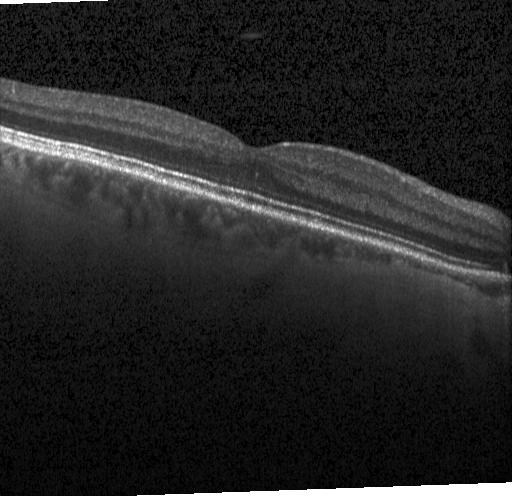
OCT B-scan; centered on the fovea; spectral-domain optical coherence tomography; instrument: Heidelberg Spectralis.
The scan shows neither choroidal neovascularization, diabetic macular edema, nor drusen.